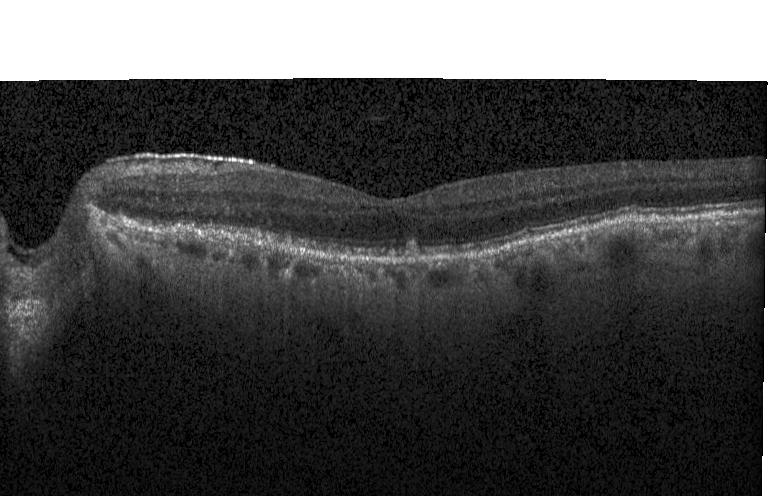

Spectral-domain OCT · horizontal scan through the fovea · retinal OCT cross-section.
Dx: multiple drusen.